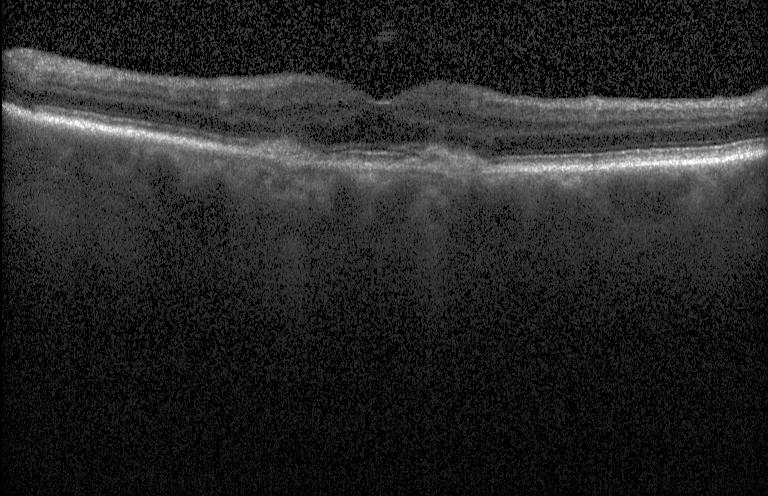

Optical coherence tomography scan — The scan shows a choroidal neovascular membrane.